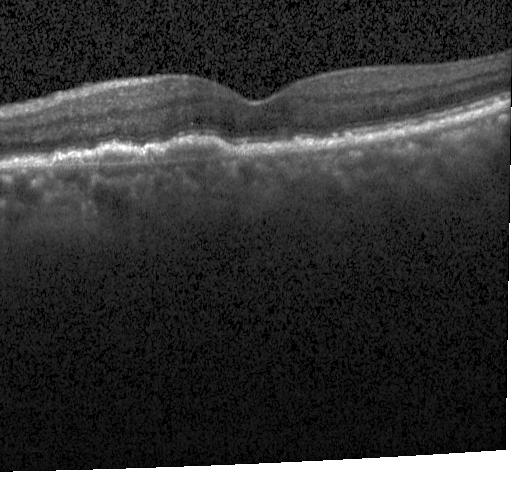 Spectral-domain OCT; optical coherence tomography scan.
The scan shows choroidal neovascularization.